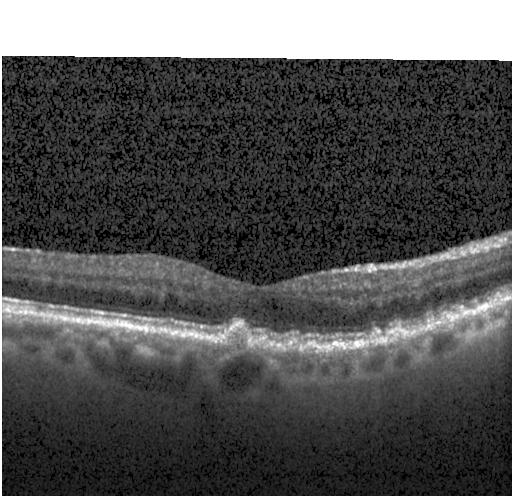 Retinal OCT cross-section
OCT finding: drusen.